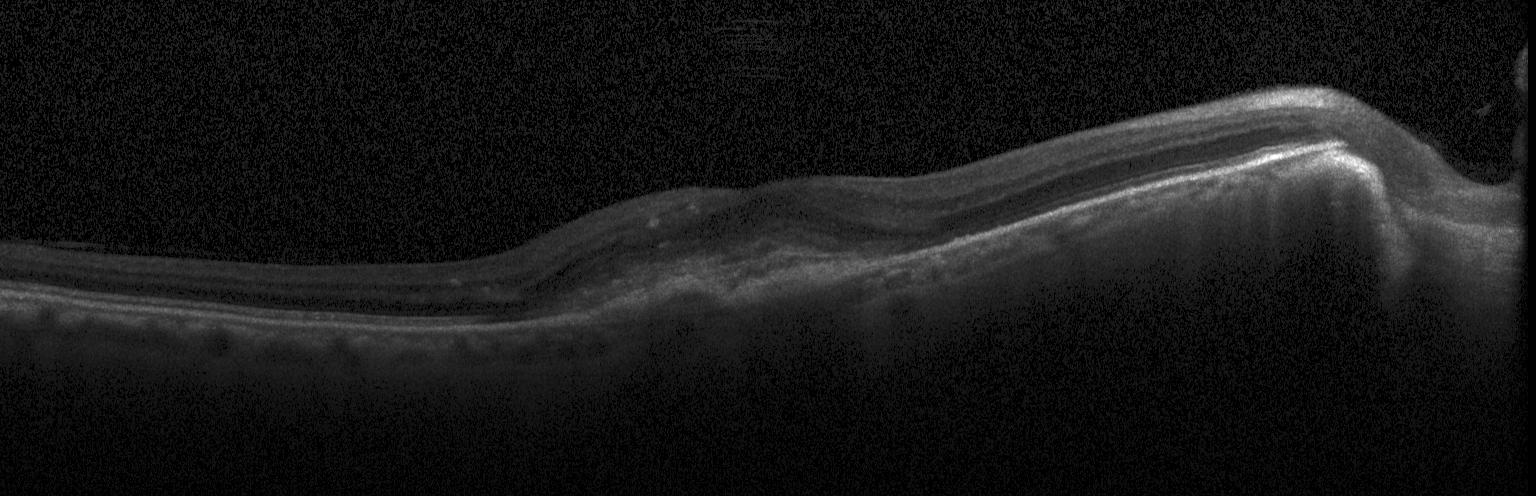 OCT scan showing a choroidal neovascular membrane.